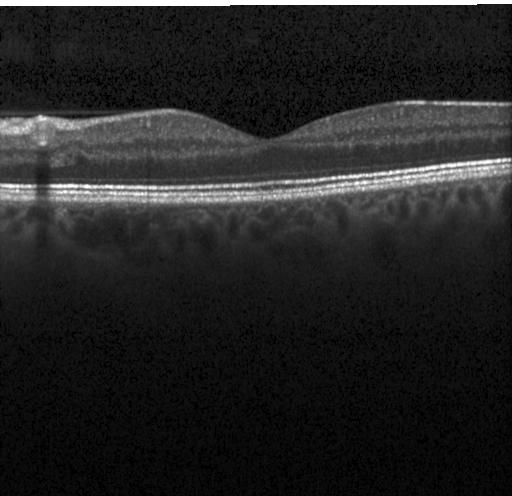 Retinal OCT cross-section, horizontal scan through the fovea.
Diagnosis: no evidence of choroidal neovascularization, diabetic macular edema, or drusen.